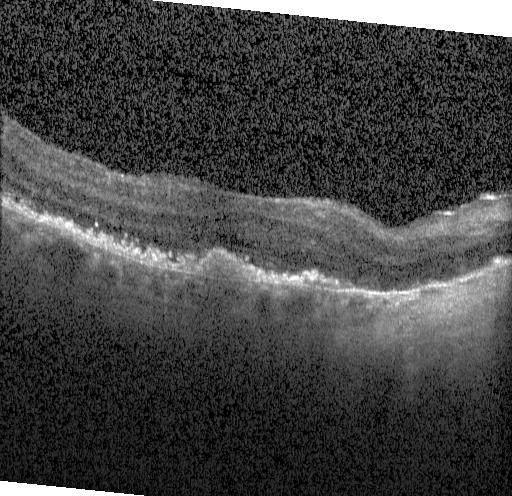
Horizontal scan through the fovea. Spectral-domain OCT. Acquired on a Heidelberg Spectralis. Optical coherence tomography scan.
This B-scan demonstrates a choroidal neovascular membrane.